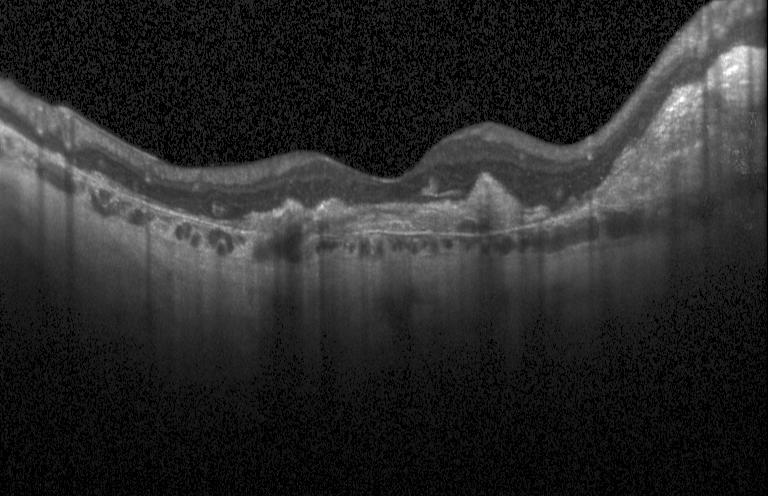

Instrument: Heidelberg Spectralis. OCT B-scan. Through the macula. SD-OCT — Assessment: CNV.